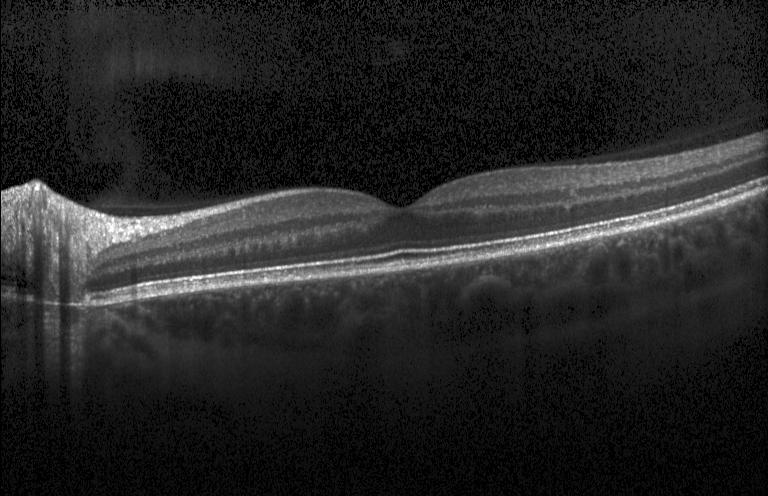 Retinal OCT cross-section showing no CNV, no DME, and no drusen.